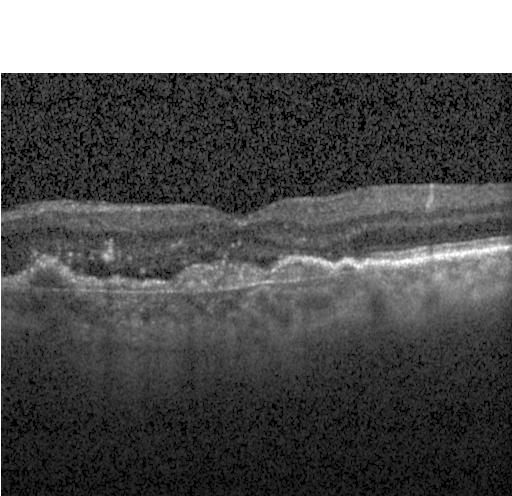 Retinal OCT cross-section.
Dx: choroidal neovascularization (CNV).